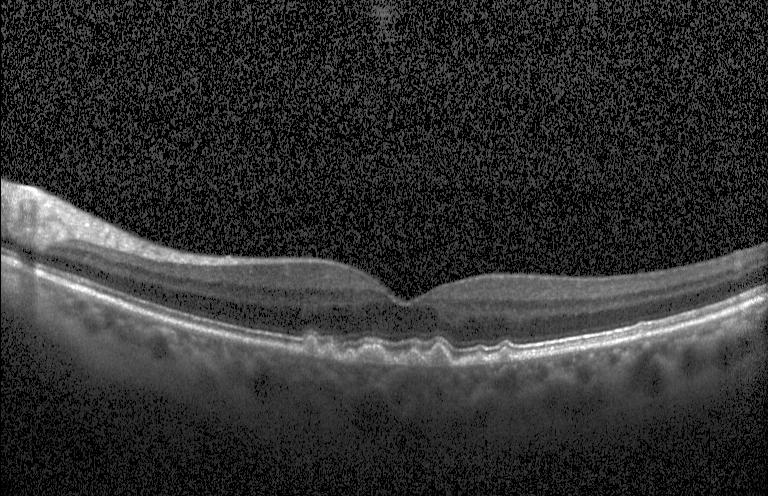

Fovea-centered; OCT line scan — Finding: sub-RPE drusenoid deposits.